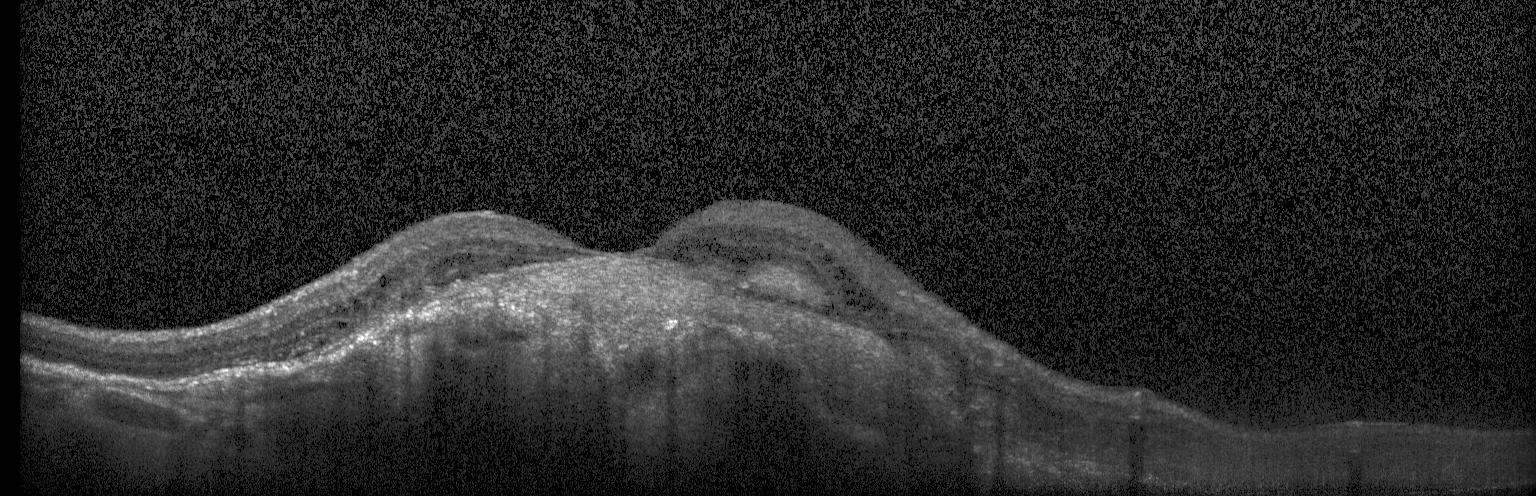

Impression: a choroidal neovascular membrane.